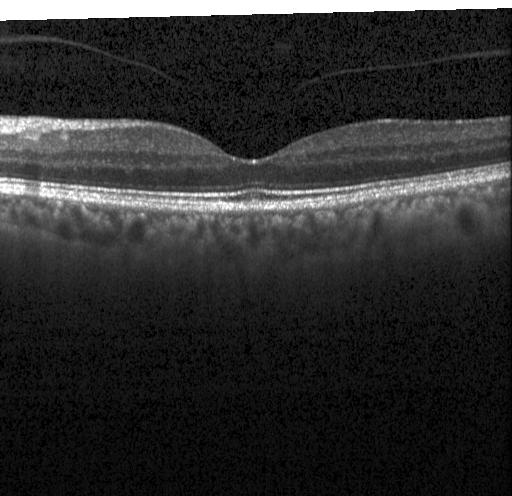

Retinal OCT cross-section
Finding: no CNV, DME, or drusen.